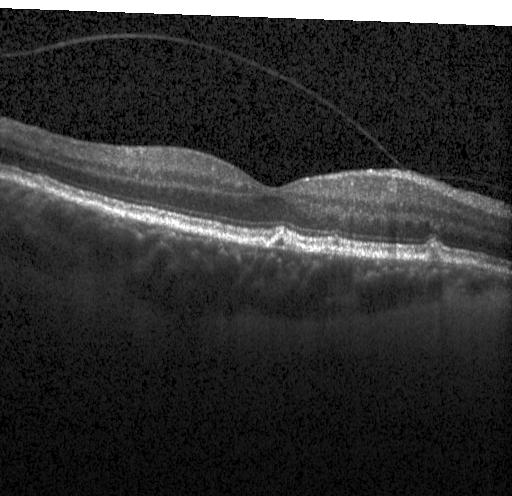
Macular OCT demonstrating sub-RPE drusenoid deposits.